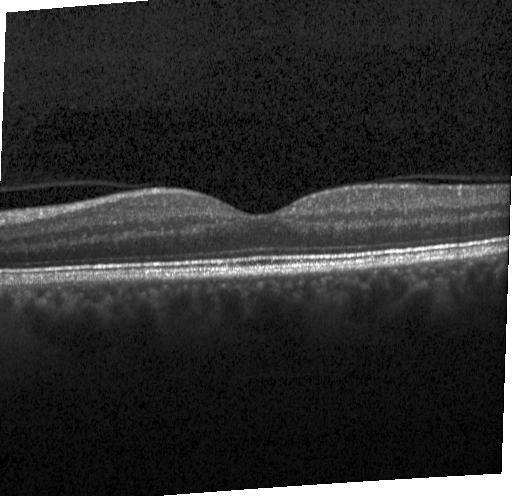
Finding: neither CNV, DME, nor drusen.